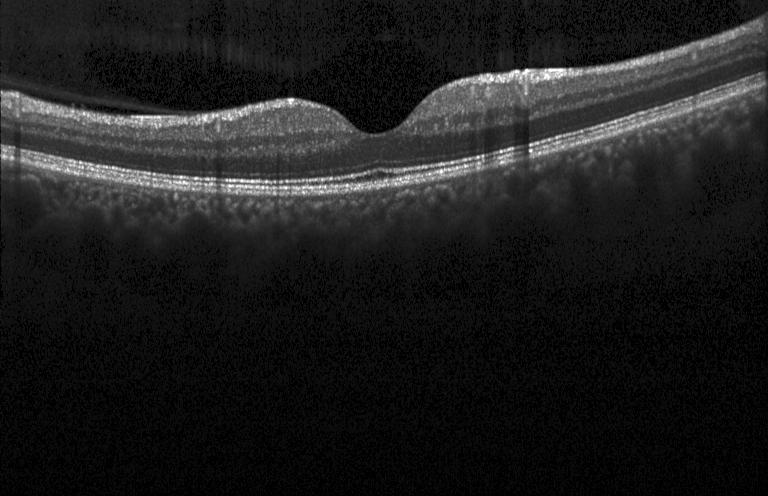

Through the macula. OCT B-scan. Heidelberg Spectralis OCT system. SD-OCT. Diagnosis: no choroidal neovascularization, no diabetic macular edema, and no drusen.